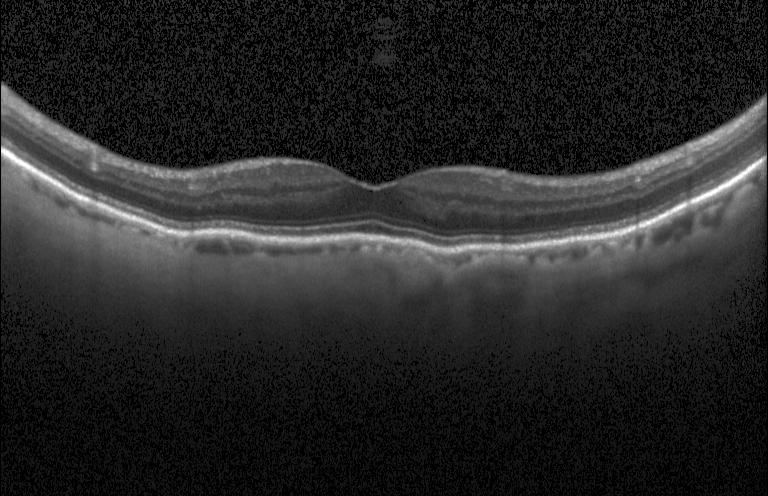
Dx: no evidence of choroidal neovascularization, diabetic macular edema, or drusen.